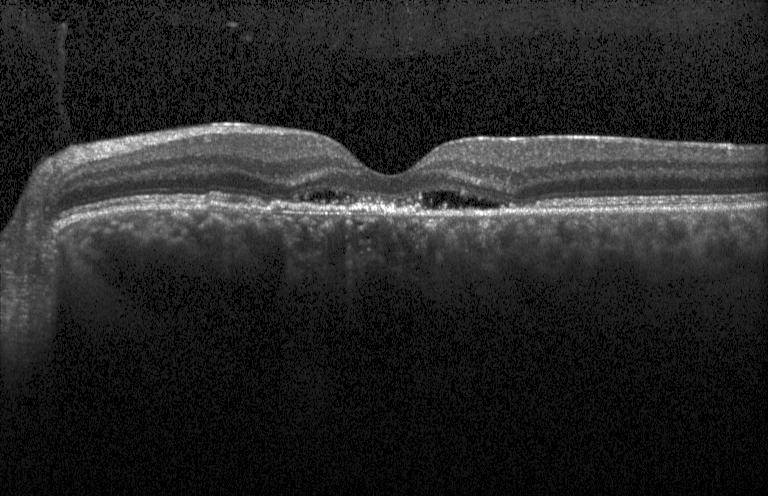

Diagnosis: a choroidal neovascular membrane.